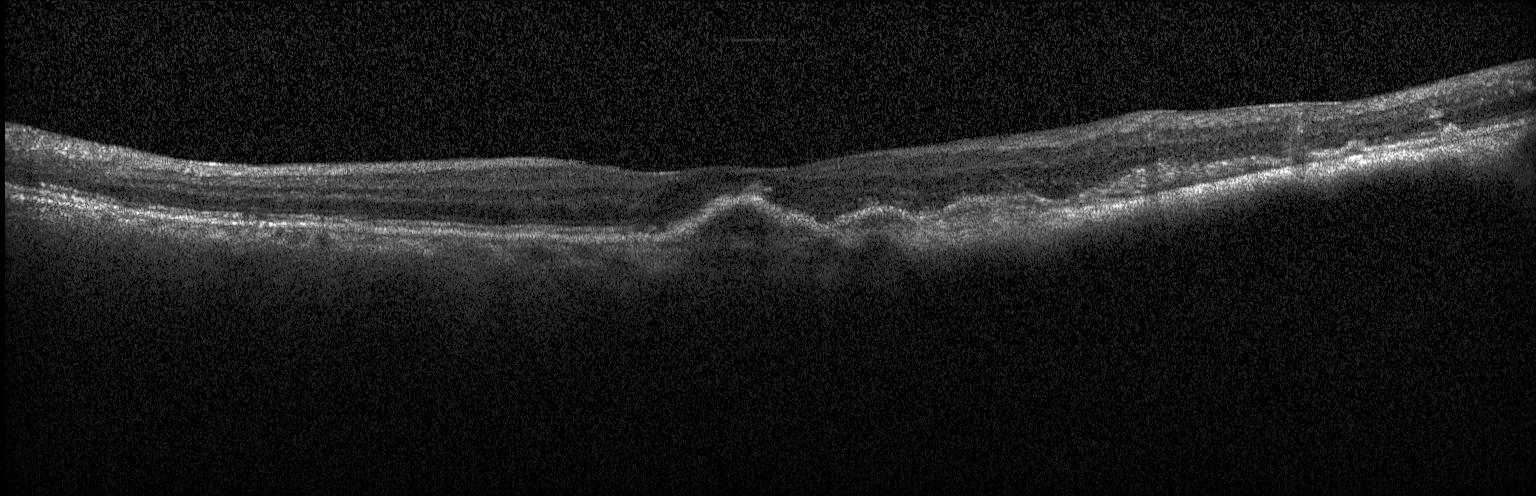 Centered on the fovea · optical coherence tomography scan · Heidelberg Spectralis OCT system — Diagnosis: CNV.